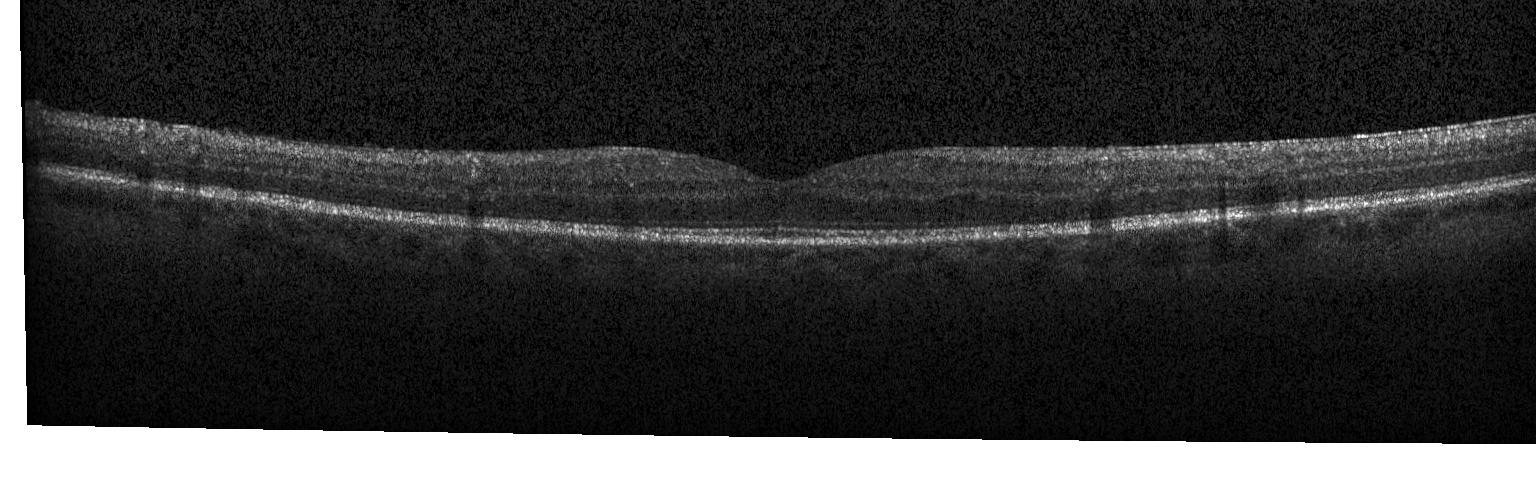 Spectral-domain OCT · acquired on a Heidelberg Spectralis · optical coherence tomography scan.
Finding: no choroidal neovascularization, no diabetic macular edema, and no drusen.